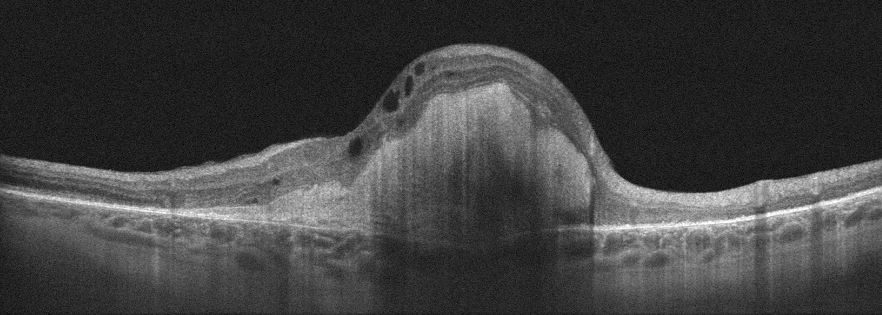
OCT B-scan, right eye. Finding: age-related macular degeneration (AMD).